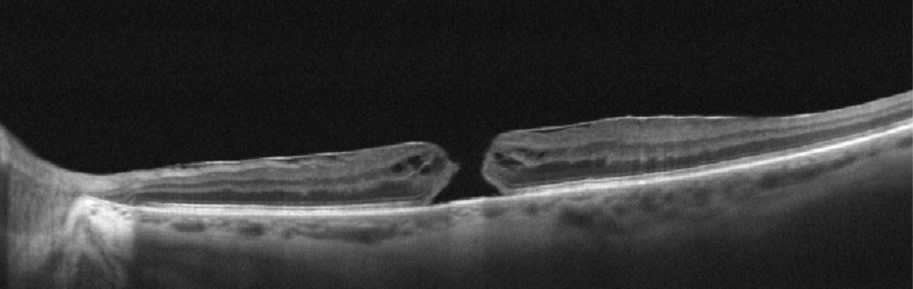

Dx: VID.